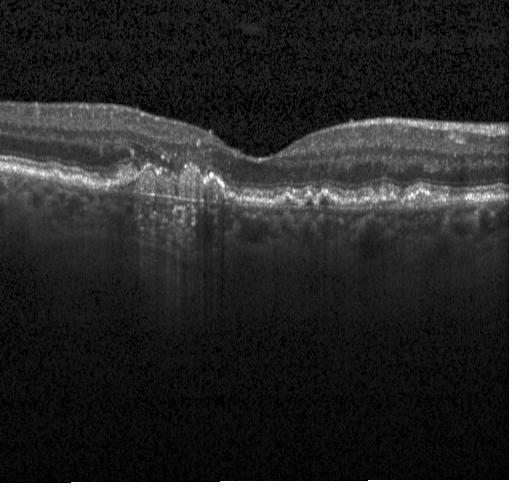
Optical coherence tomography B-scan; through the macula; Heidelberg Spectralis OCT system; spectral-domain OCT. Impression: CNV.